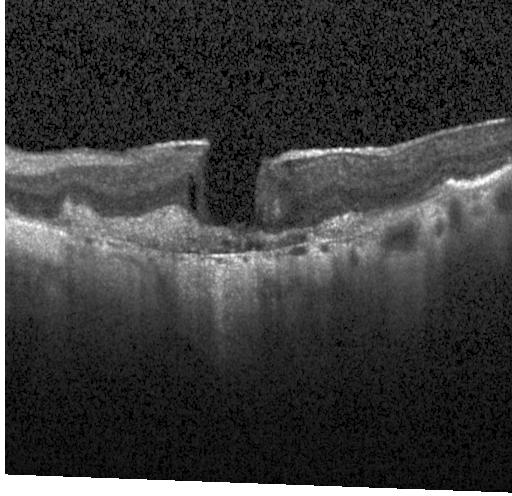

Through the macula, SD-OCT, OCT line scan.
A choroidal neovascular membrane.